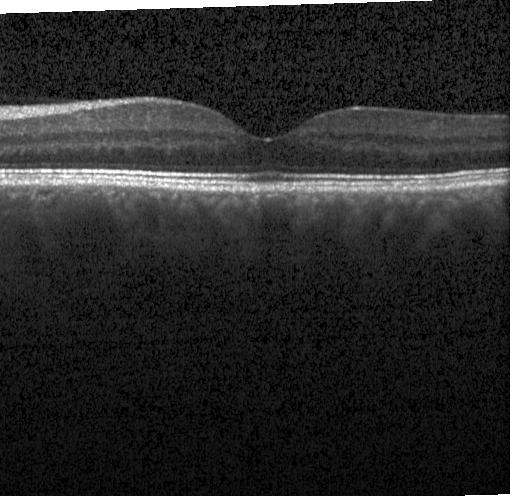 Centered on the fovea, Heidelberg Spectralis, spectral-domain optical coherence tomography, retinal OCT B-scan — Diagnosis: no evidence of CNV, DME, or drusen.